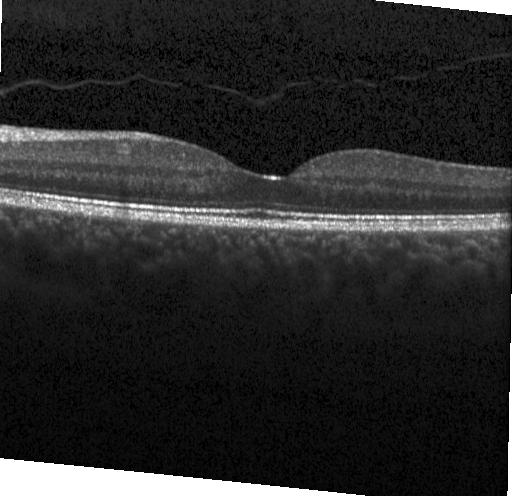

Dx: no choroidal neovascularization, no diabetic macular edema, and no drusen.